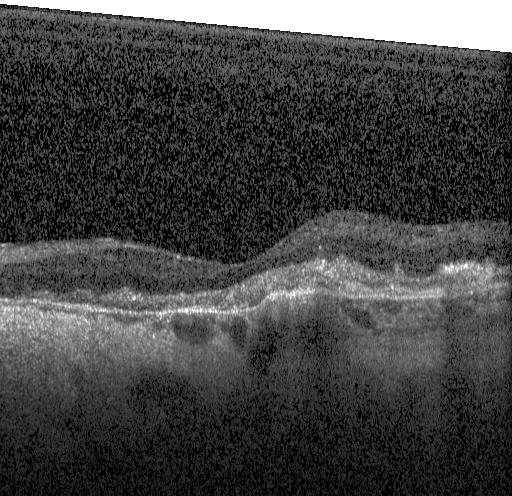 Diagnosis: a choroidal neovascular membrane.